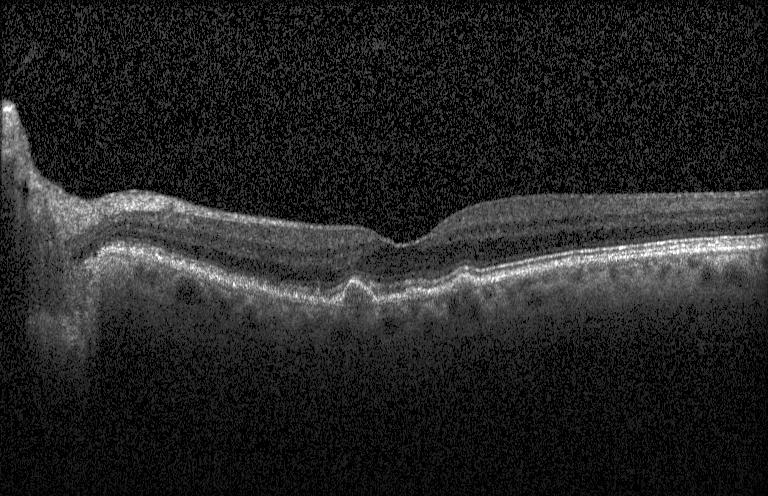

Spectral-domain optical coherence tomography, Heidelberg Spectralis OCT system, retinal OCT B-scan
Diagnosis: multiple drusen.